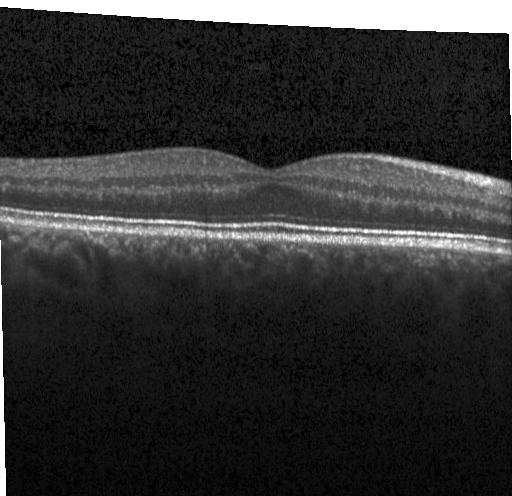

Finding: no choroidal neovascularization, no diabetic macular edema, and no drusen.